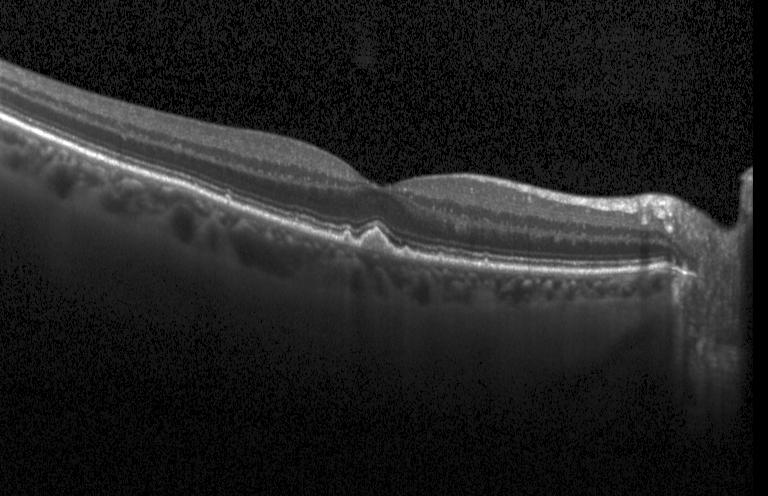

Retinal OCT B-scan.
Assessment: drusen.